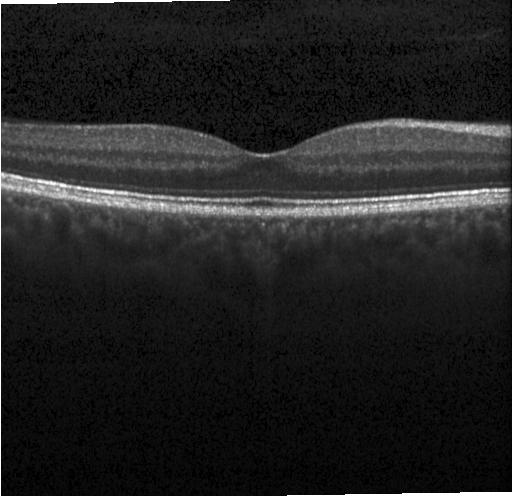

OCT finding: neither CNV, DME, nor drusen.